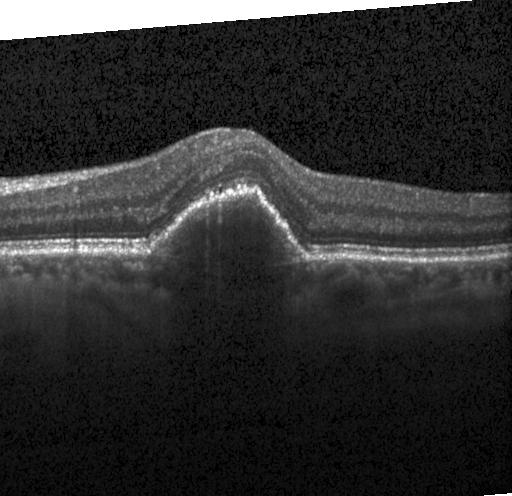 Dx: choroidal neovascularization (CNV).